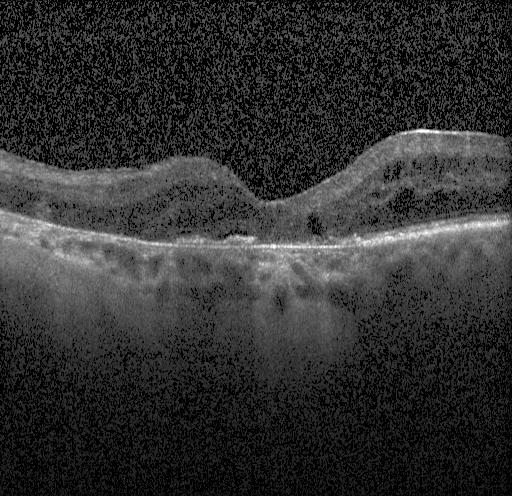
Dx: choroidal neovascularization.